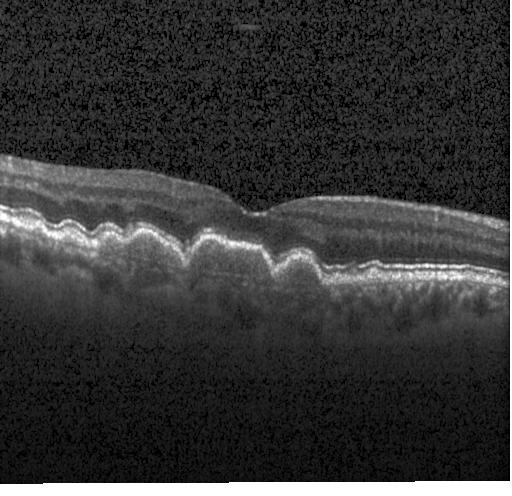
OCT line scan — OCT finding: drusen.